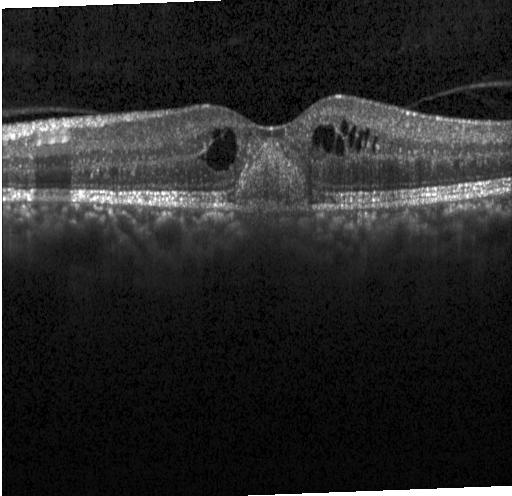
Assessment: a choroidal neovascular membrane.